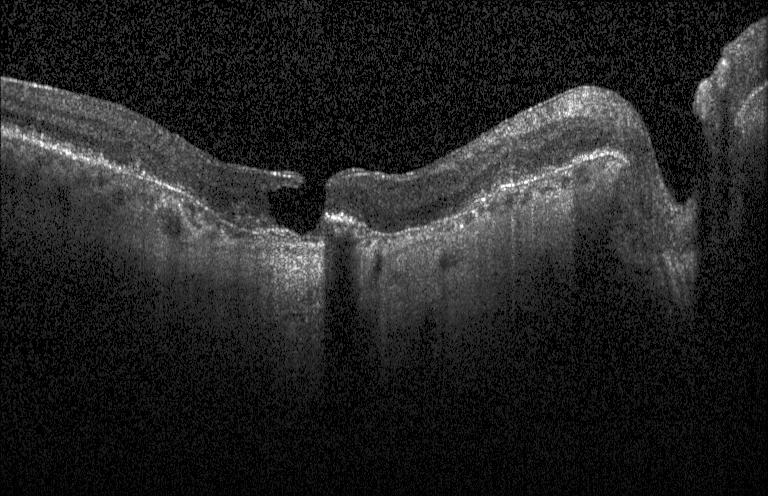 Retinal OCT cross-section showing CNV.